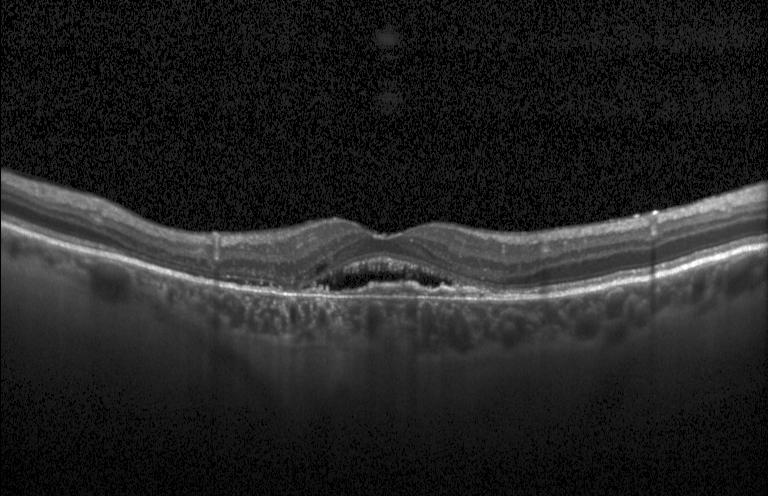

Instrument: Heidelberg Spectralis; OCT B-scan; SD-OCT. Finding: a choroidal neovascular membrane.